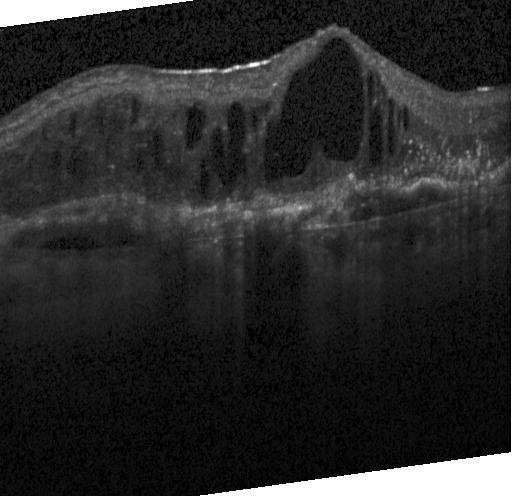 Choroidal neovascularization (CNV).